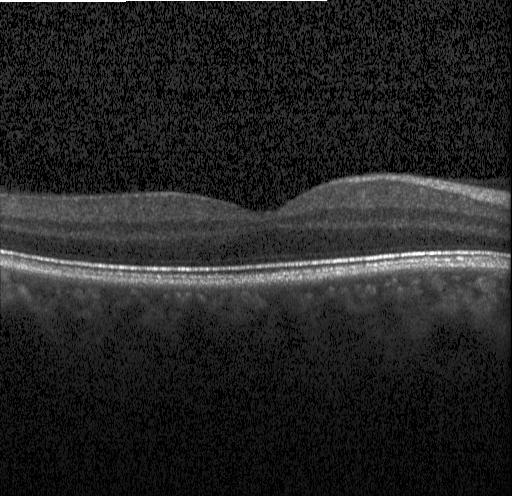 Optical coherence tomography B-scan, Heidelberg Spectralis OCT system, spectral-domain optical coherence tomography, fovea-centered
Impression: no evidence of CNV, DME, or drusen.